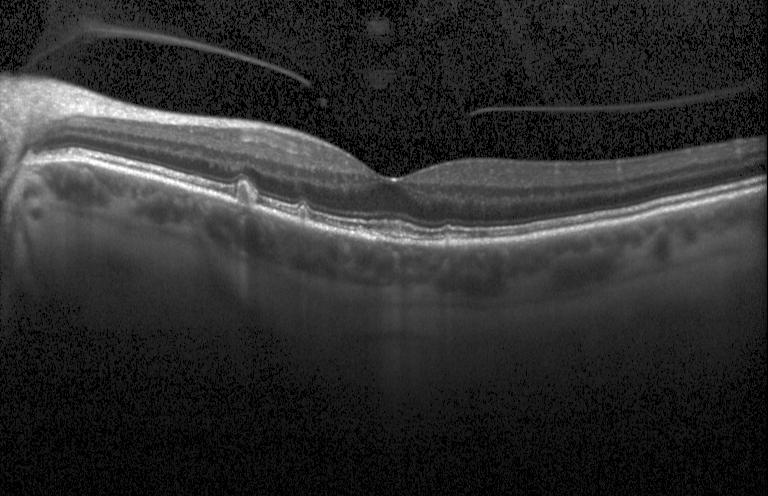
OCT B-scan — Finding: drusen.